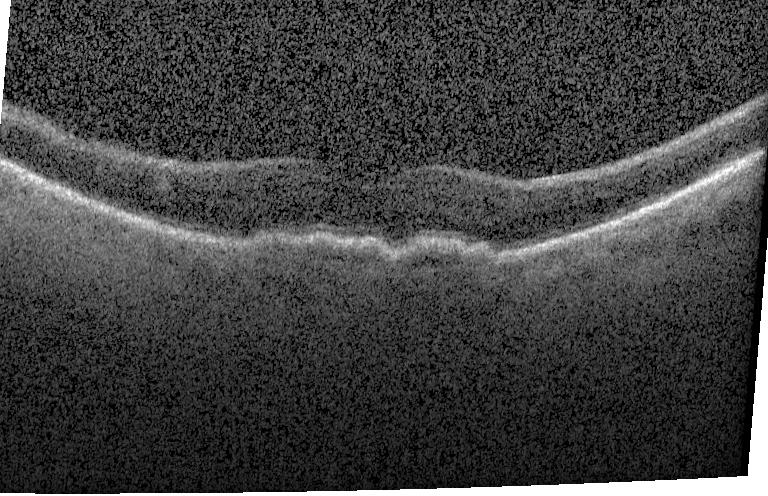

Optical coherence tomography scan · spectral-domain OCT · horizontal scan through the fovea — A choroidal neovascular membrane.